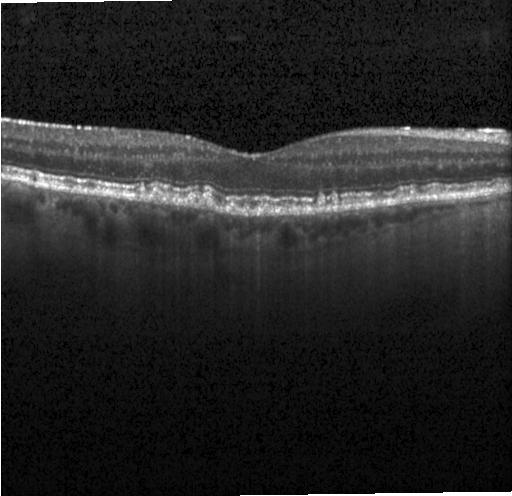
OCT finding: sub-RPE drusenoid deposits.